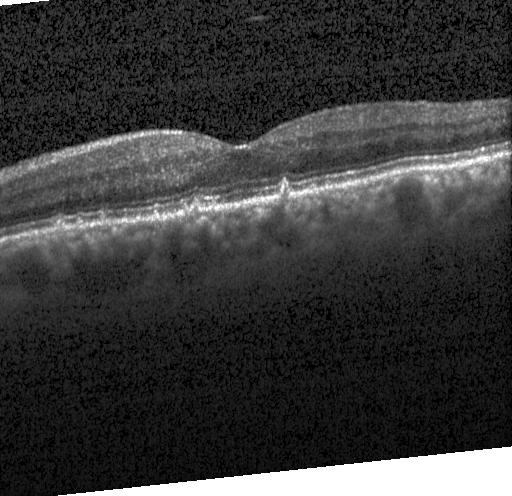 Impression: drusen.